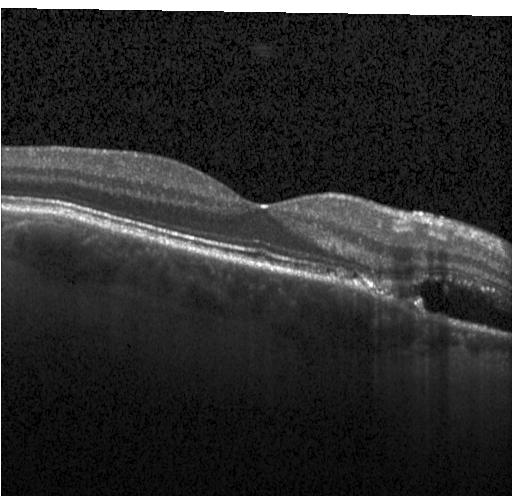

Spectral-domain optical coherence tomography; Heidelberg Spectralis OCT system; retinal OCT cross-section; through the macula.
The scan shows CNV.